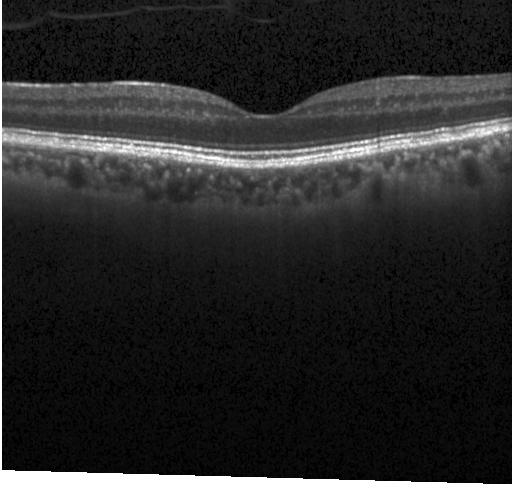
The scan shows no choroidal neovascularization, diabetic macular edema, or drusen.